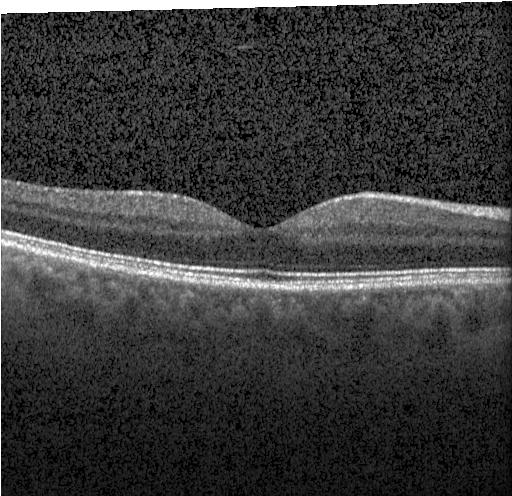 Spectral-domain OCT; OCT line scan; fovea-centered; instrument: Heidelberg Spectralis. Assessment: no evidence of choroidal neovascularization, diabetic macular edema, or drusen.